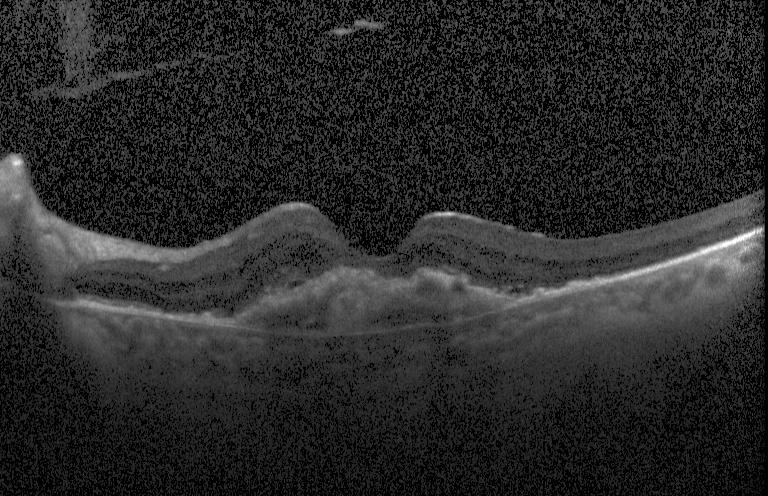
Horizontal scan through the fovea, acquired on a Heidelberg Spectralis, optical coherence tomography B-scan. Diagnosis: a choroidal neovascular membrane.